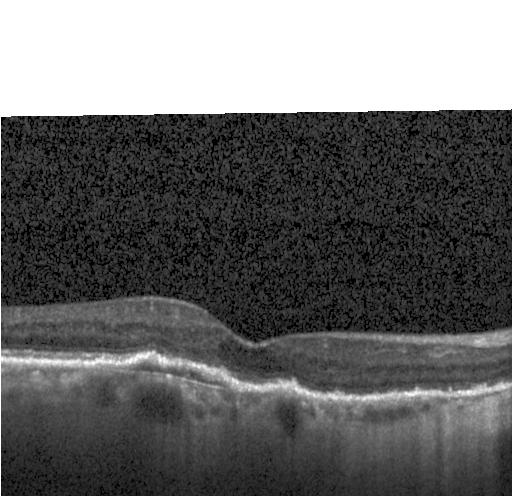

Heidelberg Spectralis OCT system; macular scan; optical coherence tomography B-scan.
Finding: a choroidal neovascular membrane.